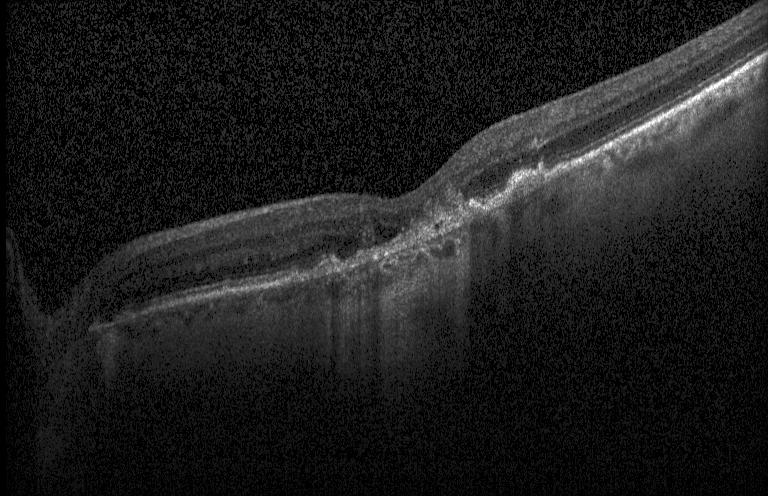
Acquired on a Heidelberg Spectralis · horizontal scan through the fovea · optical coherence tomography scan · SD-OCT — This B-scan demonstrates a choroidal neovascular membrane.